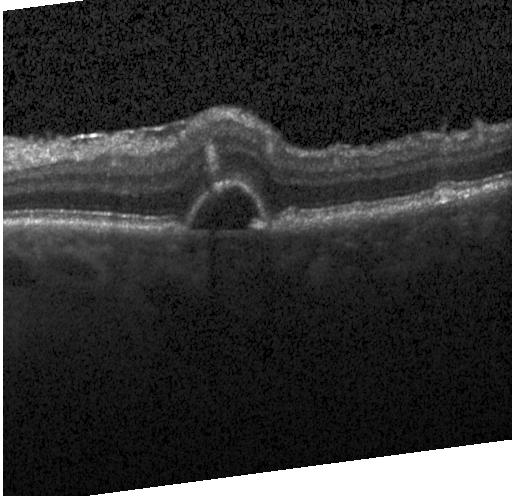

Spectral-domain OCT B-scan: a choroidal neovascular membrane.